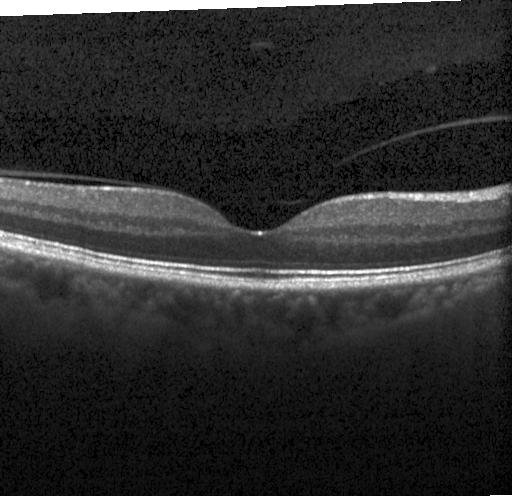

Optical coherence tomography B-scan, acquired on a Heidelberg Spectralis, spectral-domain OCT, fovea-centered — Diagnosis: no evidence of choroidal neovascularization, diabetic macular edema, or drusen.